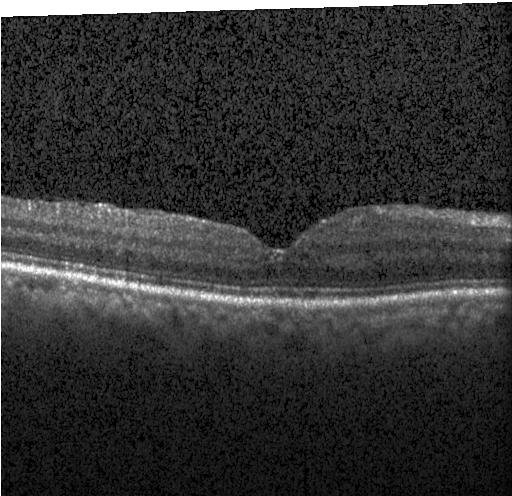 Spectral-domain OCT · horizontal scan through the fovea · optical coherence tomography scan · instrument: Heidelberg Spectralis
OCT finding: diabetic macular edema.